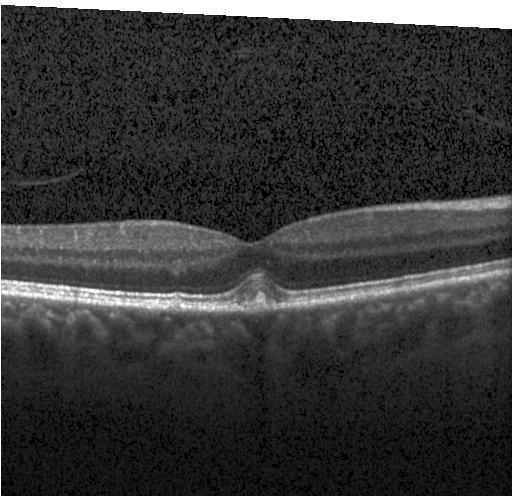
Heidelberg Spectralis OCT system. Horizontal scan through the fovea. Optical coherence tomography B-scan
Diagnosis: sub-RPE drusenoid deposits.